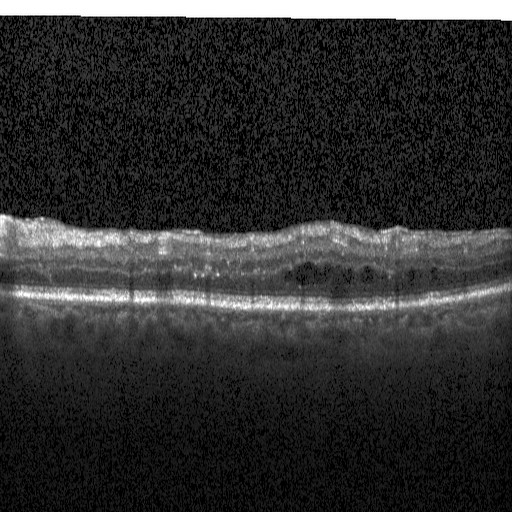 OCT line scan. Diabetic macular edema.